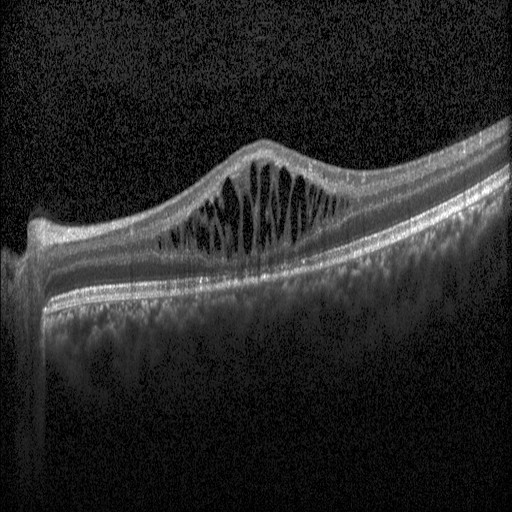
Optical coherence tomography B-scan, SD-OCT, acquired on a Heidelberg Spectralis, macular scan. The scan shows diabetic macular edema.